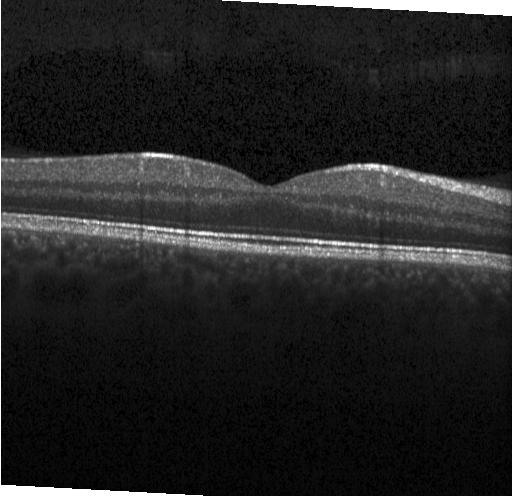

OCT line scan
Impression: no choroidal neovascularization, no diabetic macular edema, and no drusen.